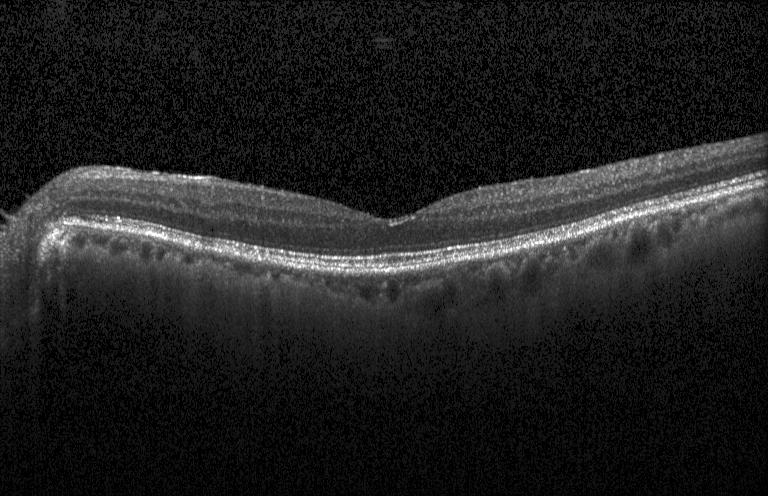

OCT B-scan; SD-OCT.
This B-scan demonstrates neither CNV, DME, nor drusen.